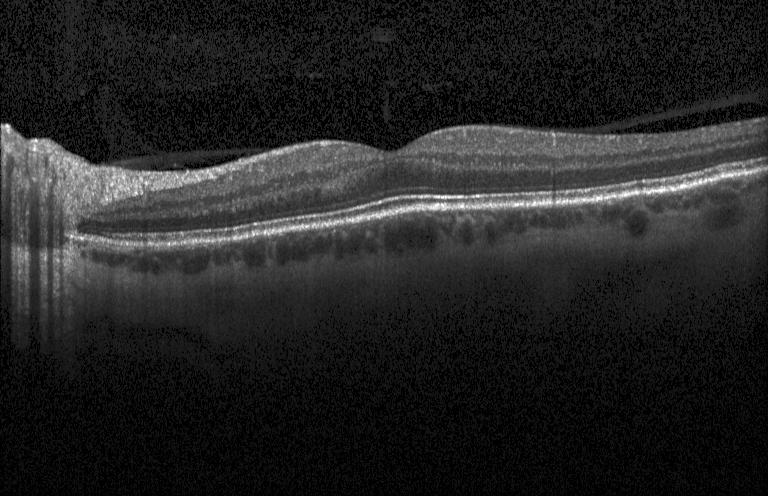

Retinal OCT B-scan.
Finding: neither CNV, DME, nor drusen.